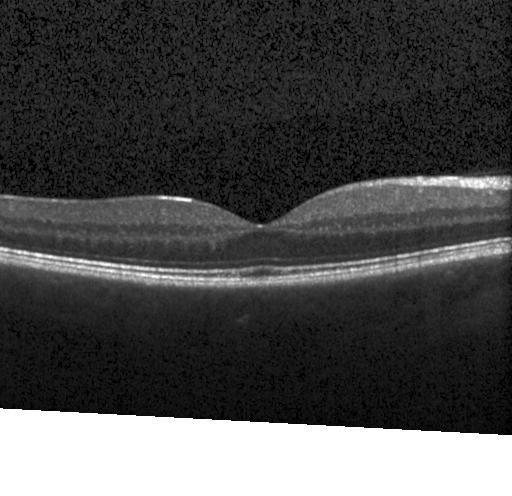 Finding: no evidence of choroidal neovascularization, diabetic macular edema, or drusen.